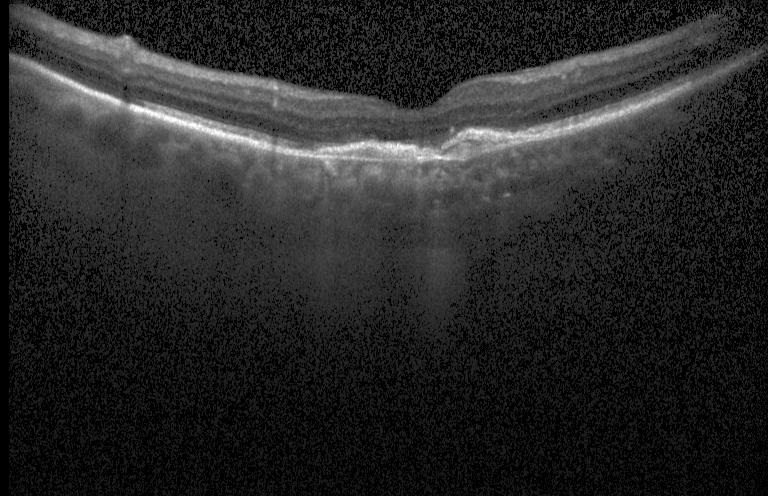 Spectral-domain OCT B-scan: choroidal neovascularization.